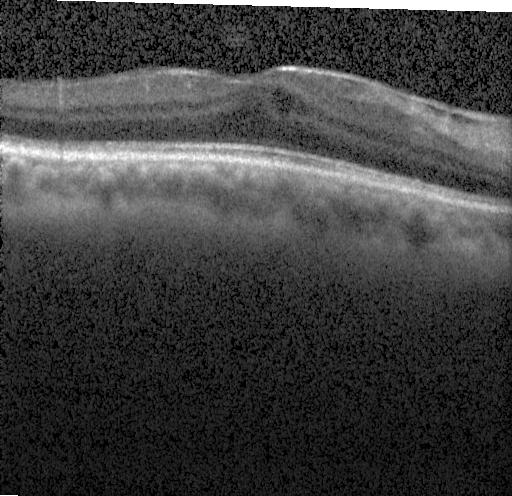

SD-OCT. Macular scan. Optical coherence tomography B-scan. Instrument: Heidelberg Spectralis.
Diagnosis: DME.